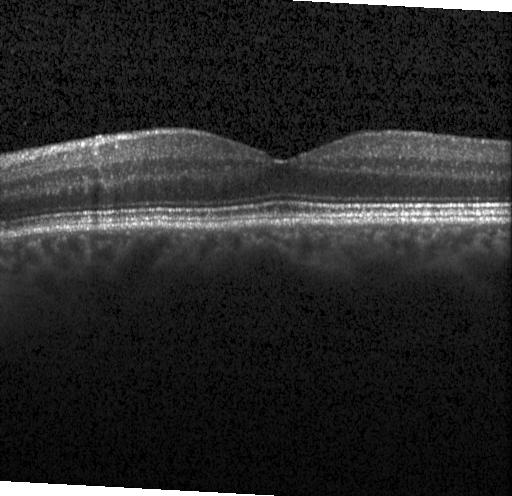 Retinal OCT B-scan; acquired on a Heidelberg Spectralis.
Finding: no evidence of choroidal neovascularization, diabetic macular edema, or drusen.